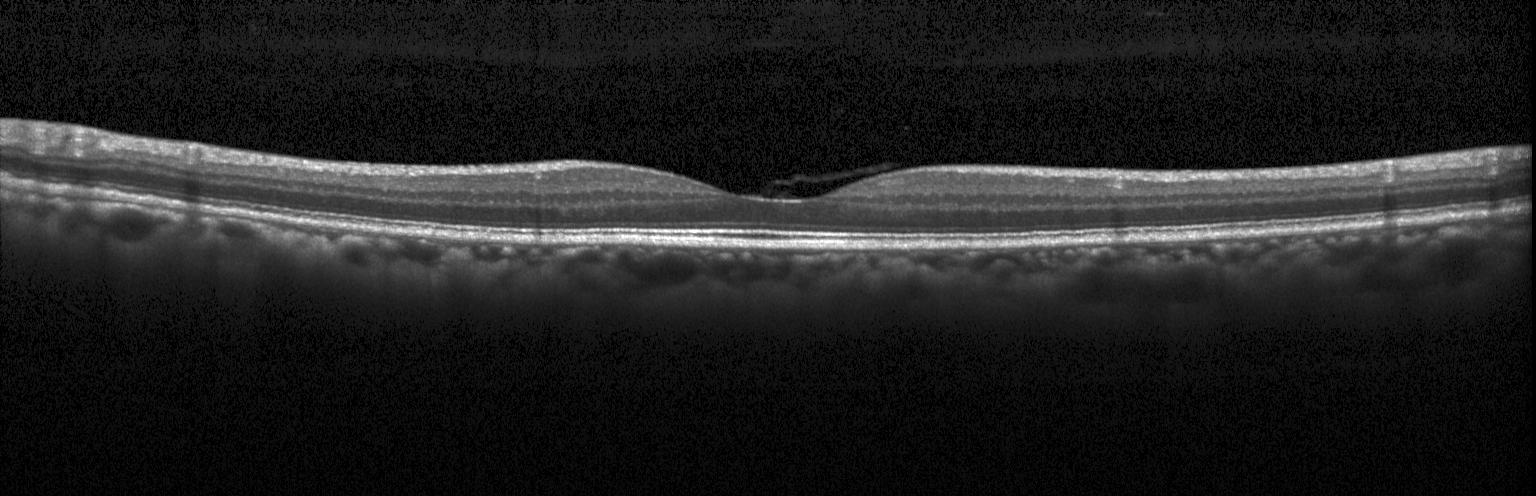 Heidelberg Spectralis · optical coherence tomography scan · centered on the fovea · SD-OCT.
Assessment: no CNV, no DME, and no drusen.